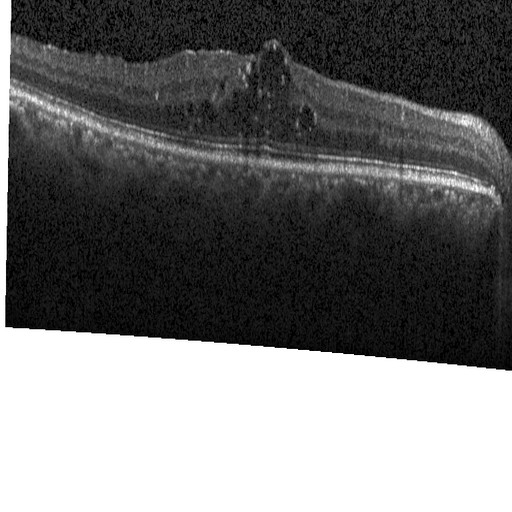

Centered on the fovea · retinal OCT B-scan.
Diagnosis: diabetic macular edema (DME).